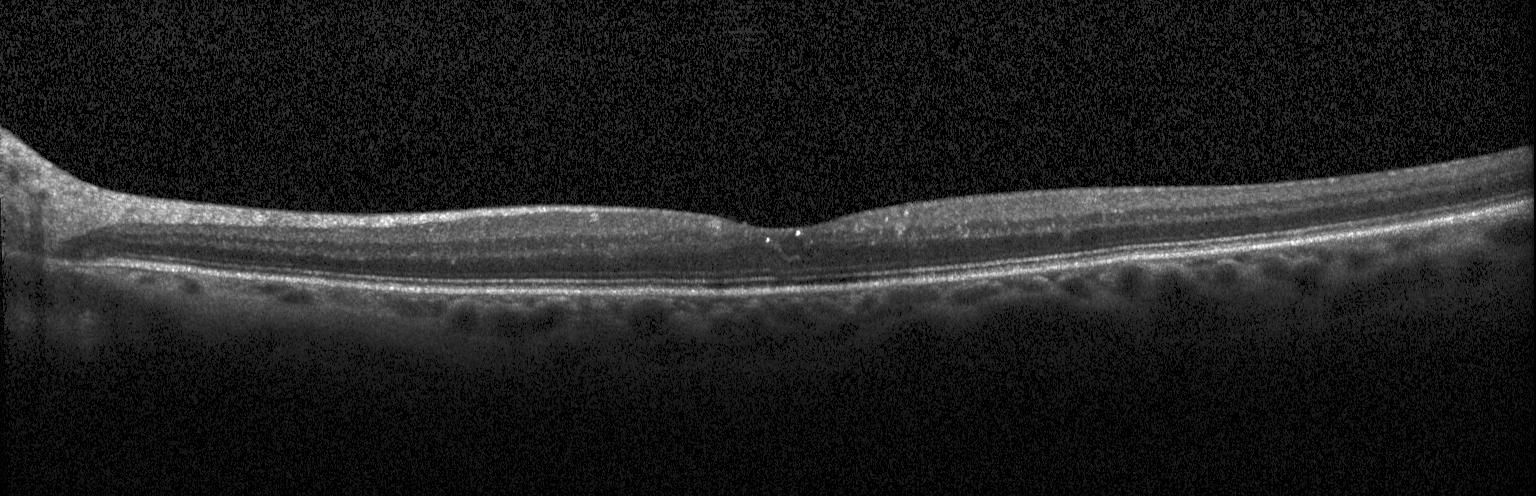 Macular scan, retinal OCT cross-section, acquired on a Heidelberg Spectralis, SD-OCT.
The scan shows no choroidal neovascularization, diabetic macular edema, or drusen.